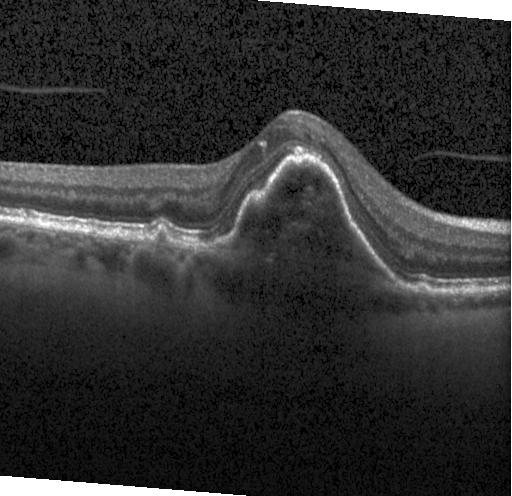 Optical coherence tomography B-scan. Assessment: a choroidal neovascular membrane.